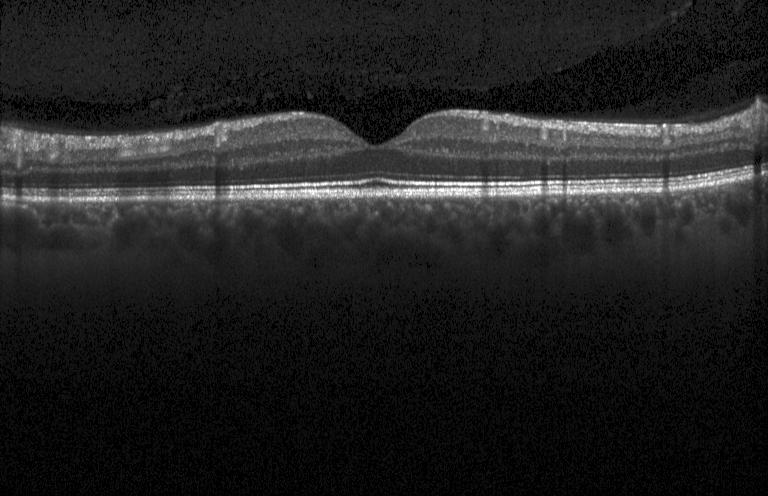

Optical coherence tomography B-scan. Impression: no choroidal neovascularization, diabetic macular edema, or drusen.